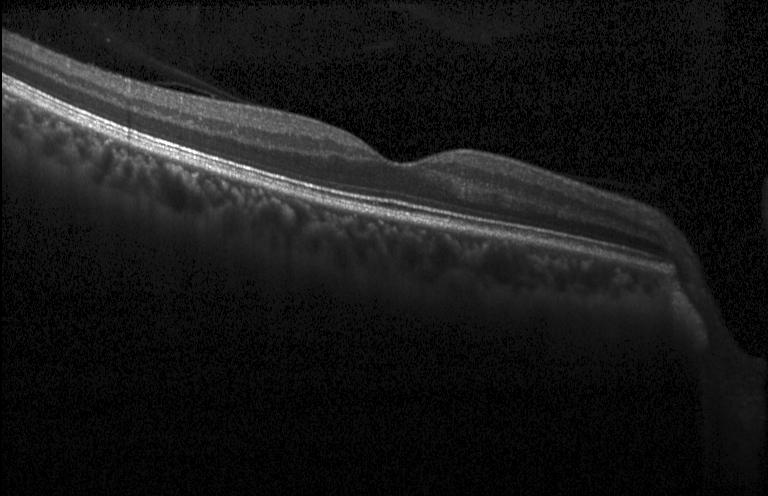 Retinal OCT cross-section showing neither CNV, DME, nor drusen.